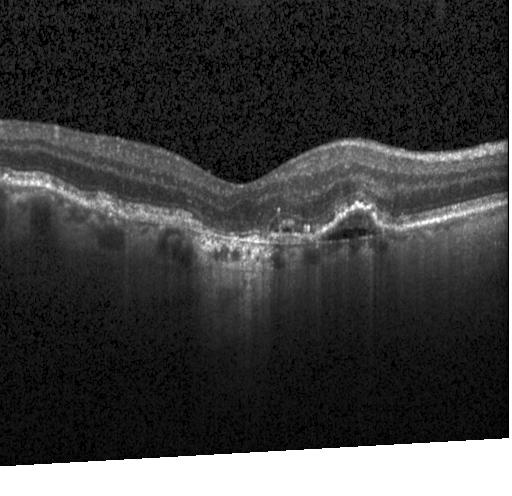 Retinal OCT cross-section. Assessment: choroidal neovascularization (CNV).